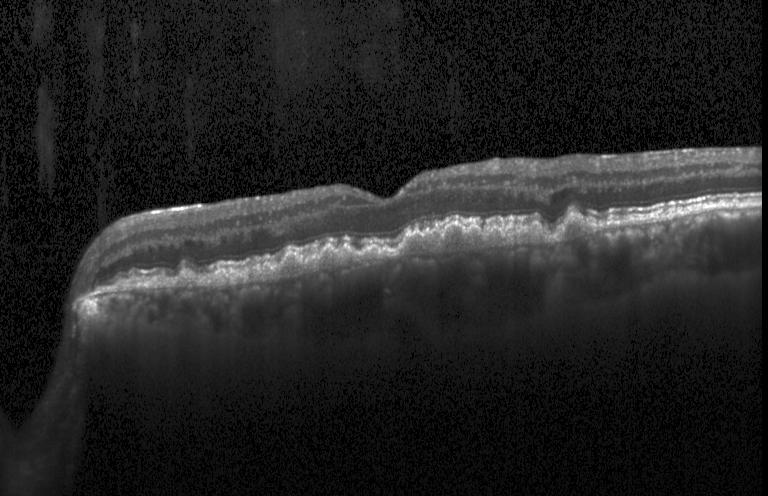
Optical coherence tomography scan — This B-scan demonstrates CNV.